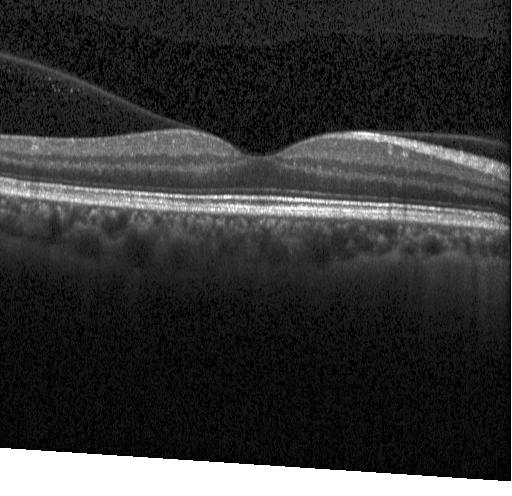

Dx: no choroidal neovascularization, diabetic macular edema, or drusen.